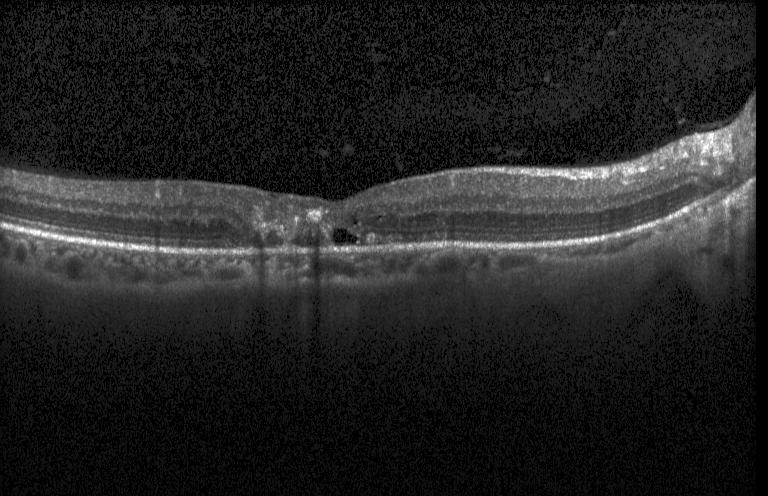 OCT B-scan showing a choroidal neovascular membrane.